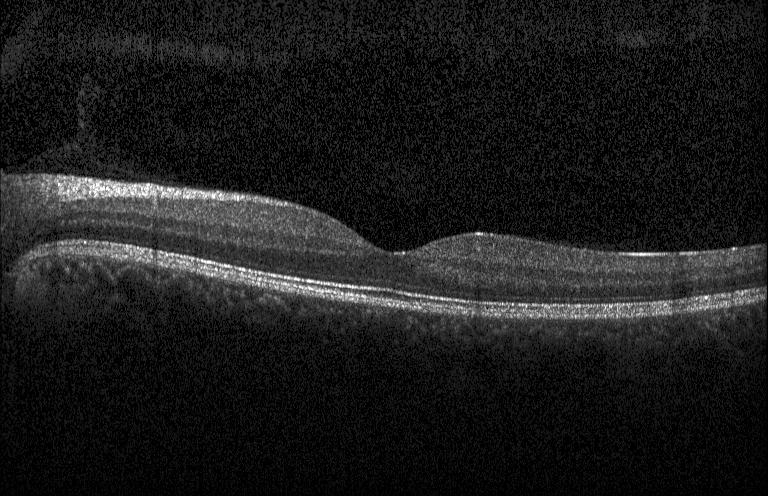
Macular OCT demonstrating no choroidal neovascularization, no diabetic macular edema, and no drusen.